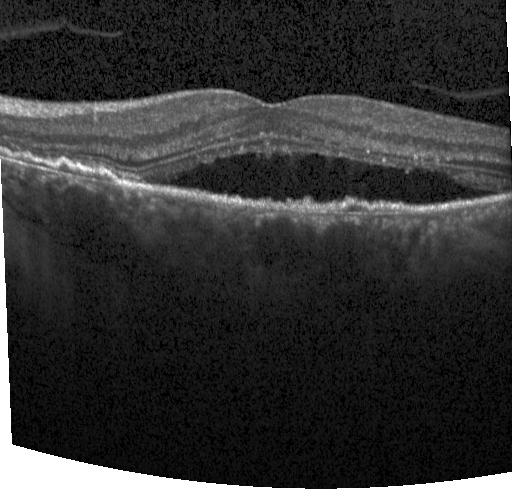 Horizontal scan through the fovea; spectral-domain OCT; Heidelberg Spectralis; retinal OCT cross-section.
Dx: a choroidal neovascular membrane.